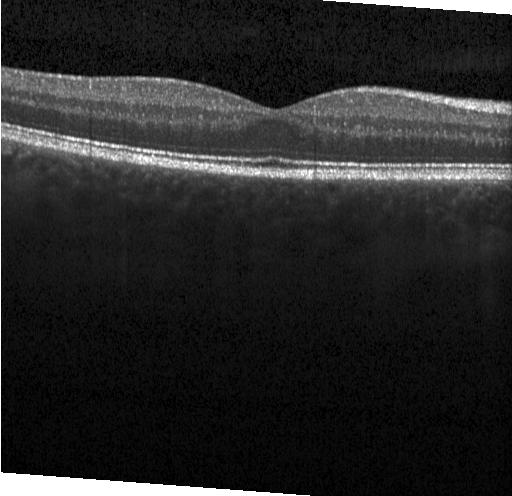
Optical coherence tomography B-scan. Assessment: no evidence of CNV, DME, or drusen.